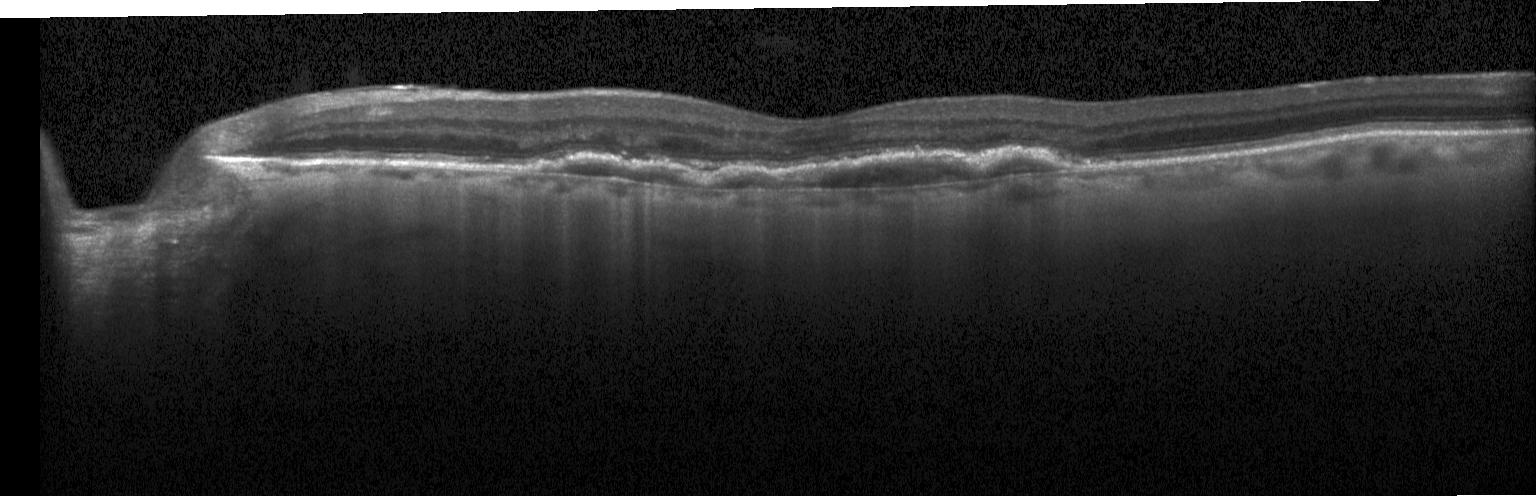
Horizontal scan through the fovea · optical coherence tomography B-scan · spectral-domain optical coherence tomography. Diagnosis: CNV.